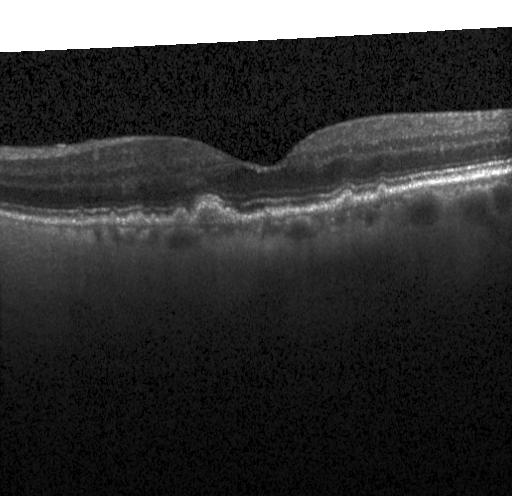 Retinal OCT B-scan. Impression: sub-RPE drusenoid deposits.